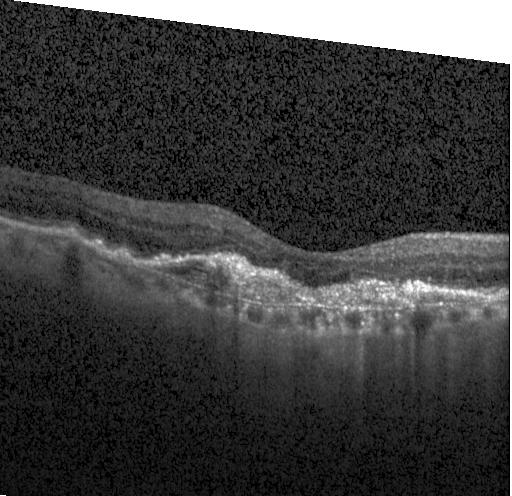
Diagnosis: a choroidal neovascular membrane.